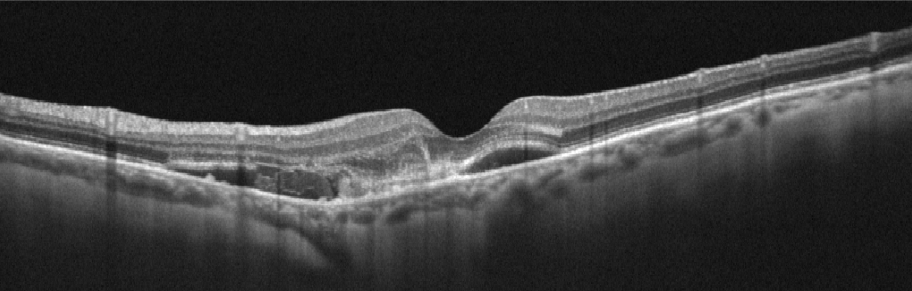

OCT B-scan
Impression: age-related macular degeneration (AMD).